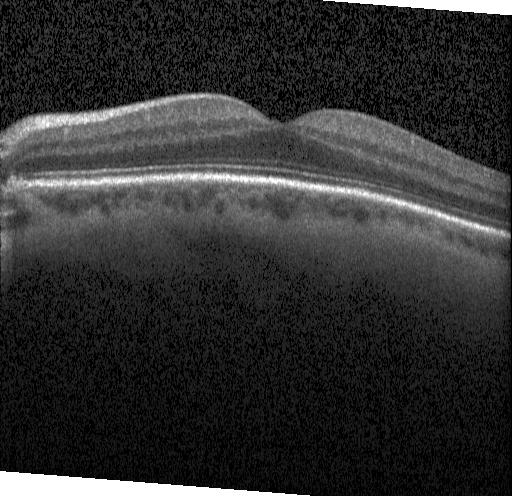
Macular OCT demonstrating no evidence of choroidal neovascularization, diabetic macular edema, or drusen.